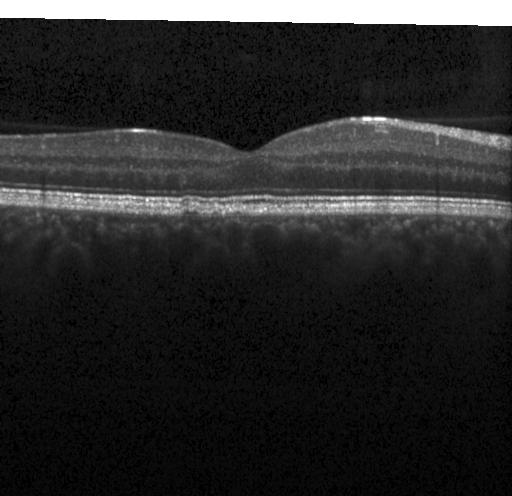 Finding: multiple drusen.